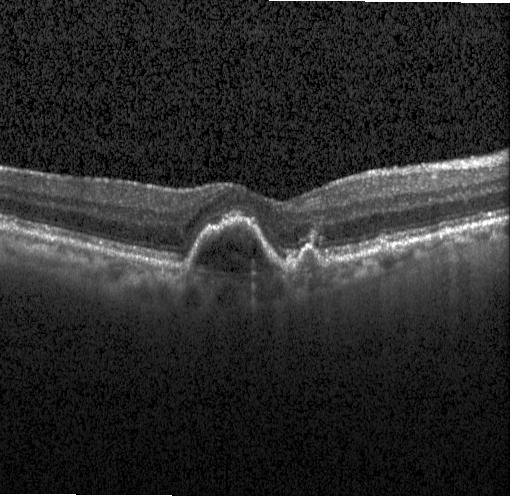 Macular OCT: choroidal neovascularization.